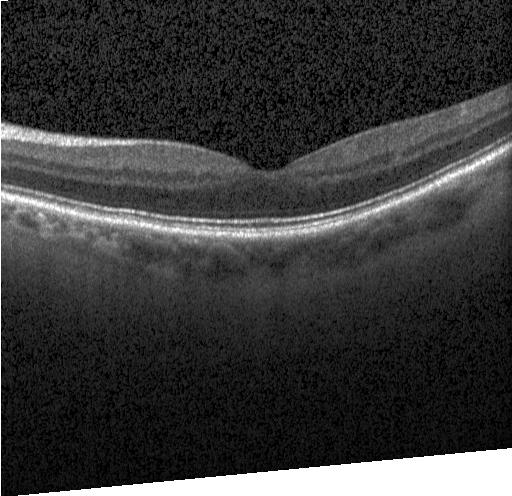
Acquired on a Heidelberg Spectralis. Fovea-centered. Optical coherence tomography scan
Dx: neither CNV, DME, nor drusen.